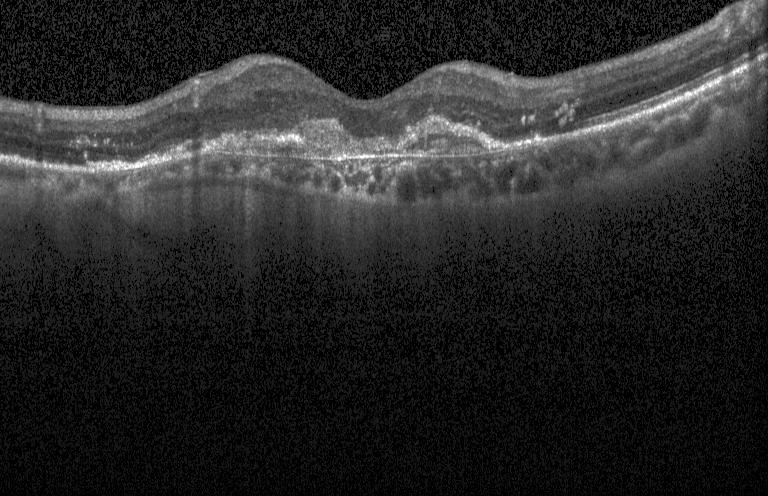
OCT finding: CNV.